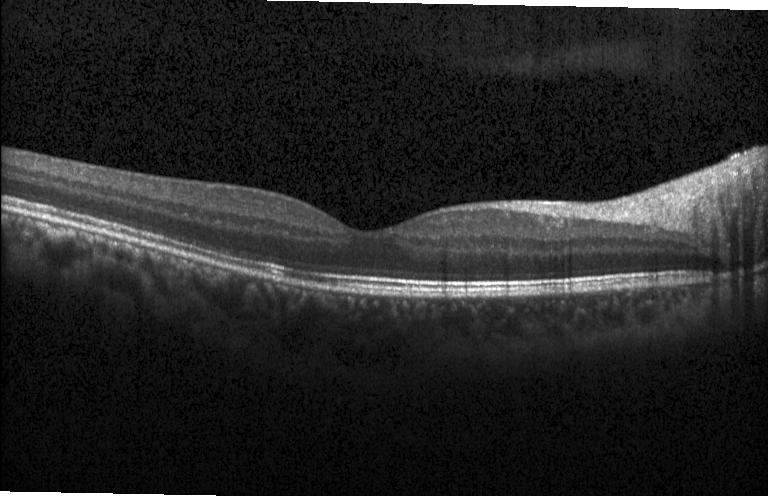

Diagnosis: no CNV, no DME, and no drusen.